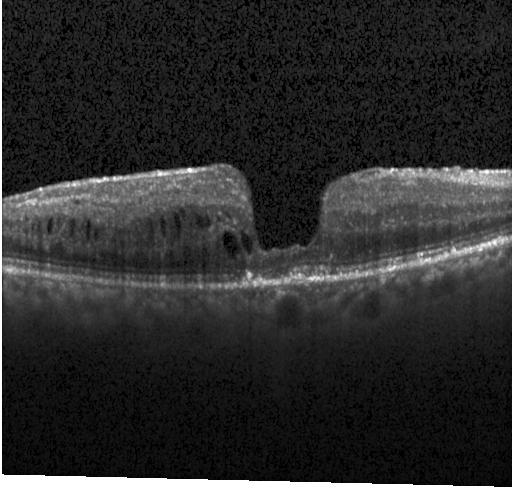
OCT B-scan · spectral-domain optical coherence tomography — Finding: diabetic macular edema.